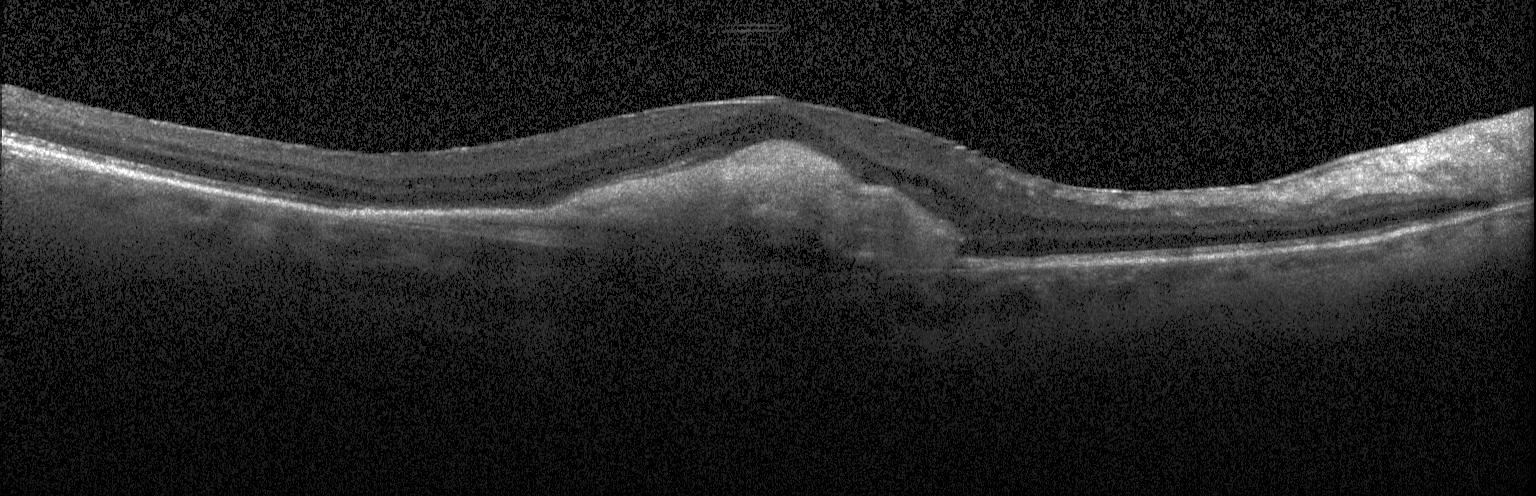

Spectral-domain optical coherence tomography. OCT B-scan. Heidelberg Spectralis — Impression: a choroidal neovascular membrane.